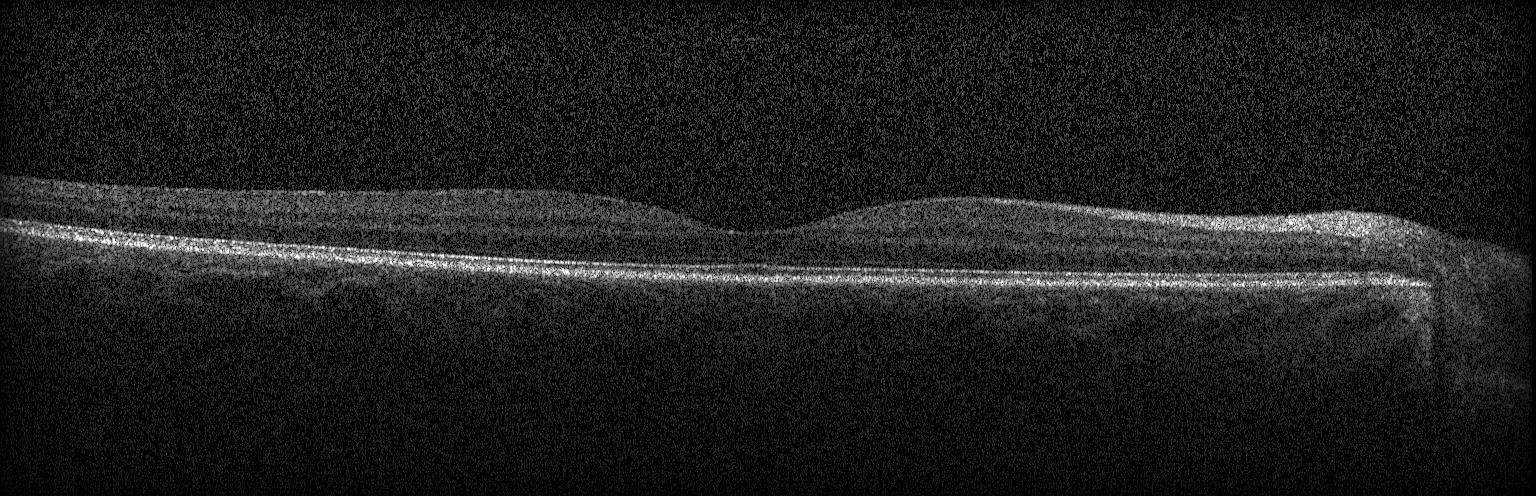
No choroidal neovascularization, diabetic macular edema, or drusen.